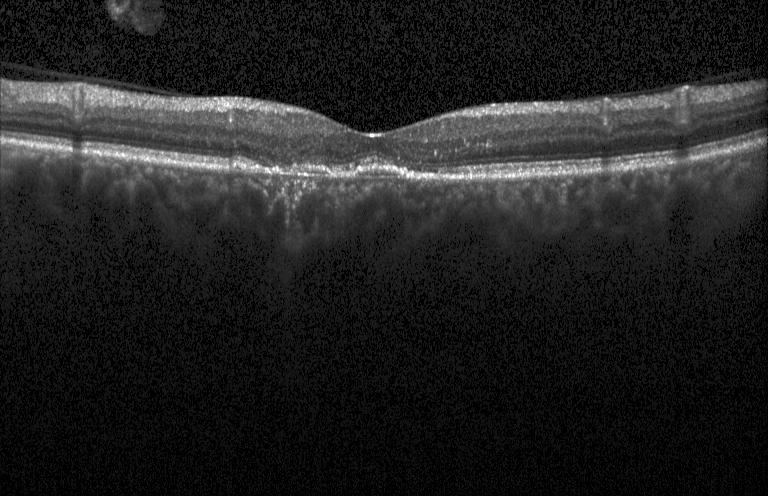
Spectral-domain OCT · retinal OCT B-scan. Finding: CNV.